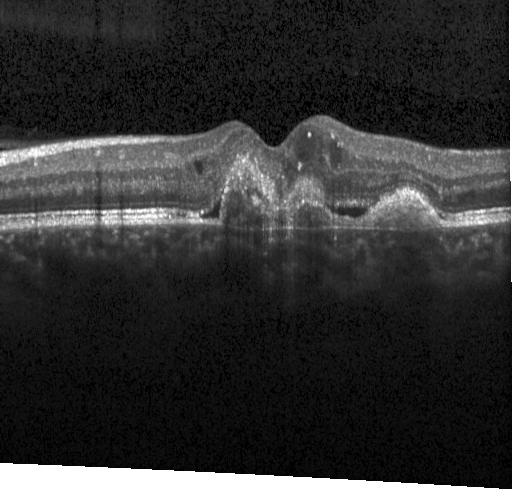

Heidelberg Spectralis · optical coherence tomography B-scan · through the macula
Finding: a choroidal neovascular membrane.